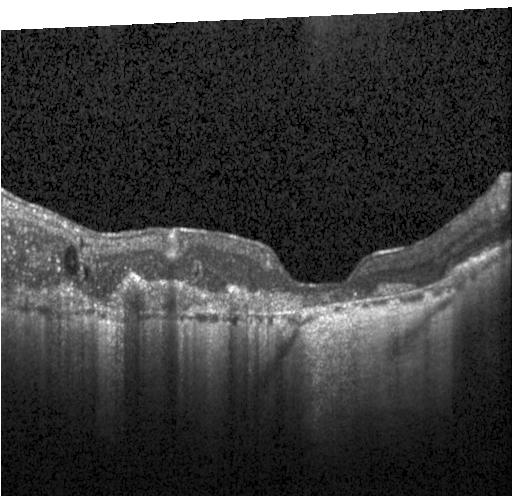 Through the macula, OCT B-scan, spectral-domain OCT
The scan shows a choroidal neovascular membrane.